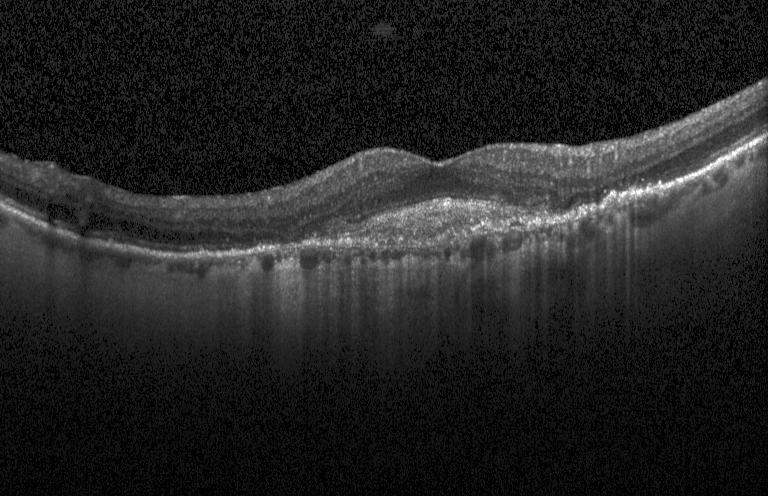

Spectral-domain optical coherence tomography. Optical coherence tomography scan. Heidelberg Spectralis. Through the macula. OCT finding: a choroidal neovascular membrane.